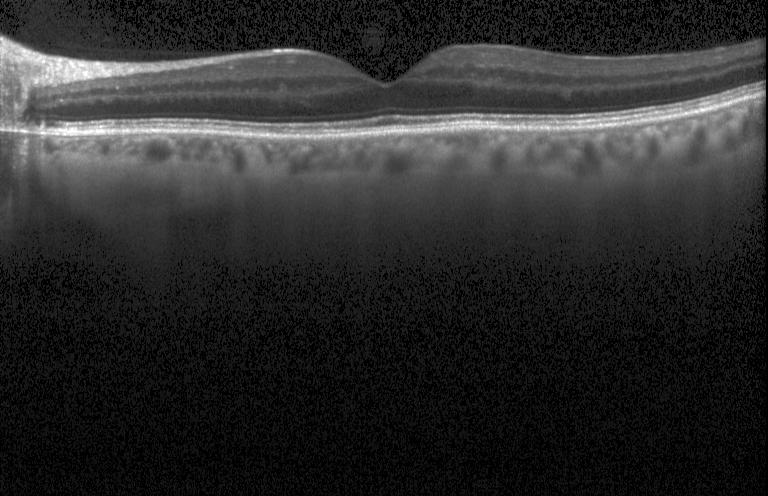
Spectral-domain optical coherence tomography · OCT B-scan.
Impression: no choroidal neovascularization, no diabetic macular edema, and no drusen.